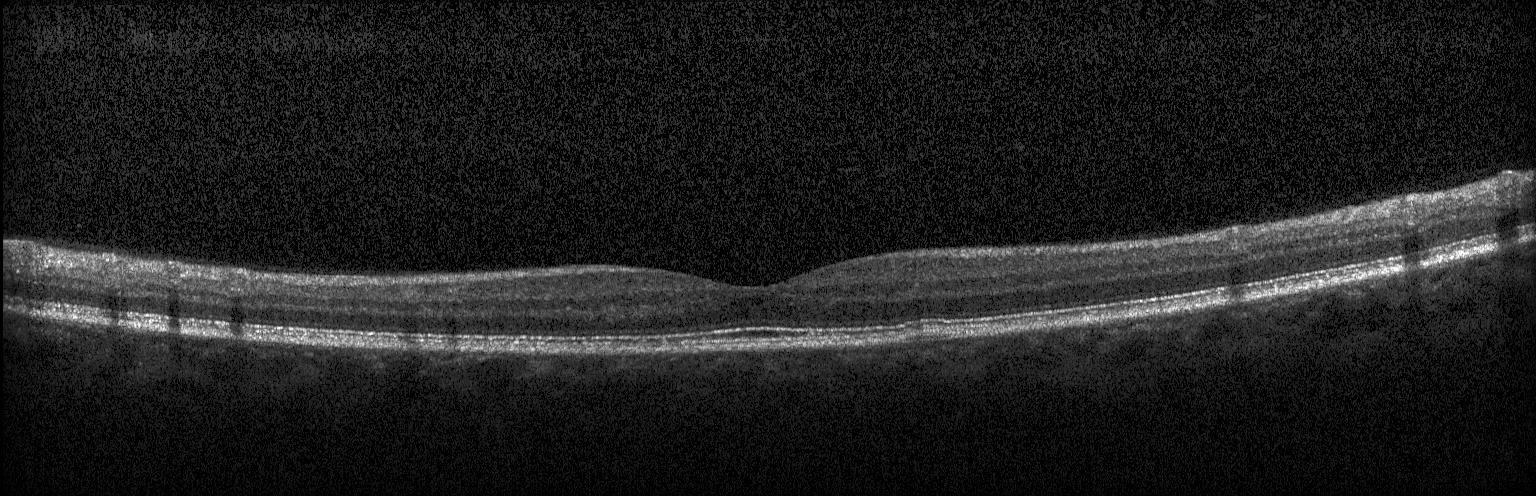 Retinal OCT cross-section
Finding: no evidence of choroidal neovascularization, diabetic macular edema, or drusen.